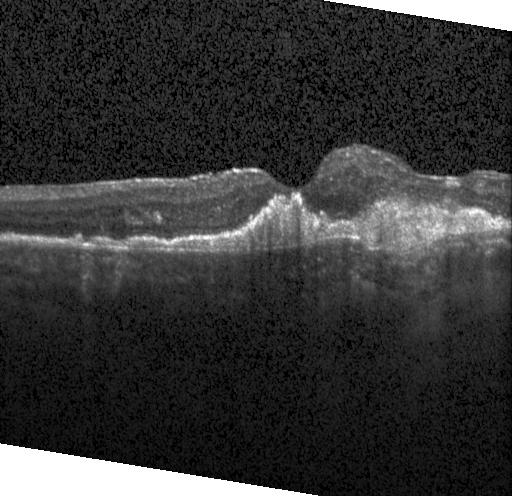 SD-OCT, horizontal scan through the fovea, OCT line scan, Heidelberg Spectralis — Impression: CNV.